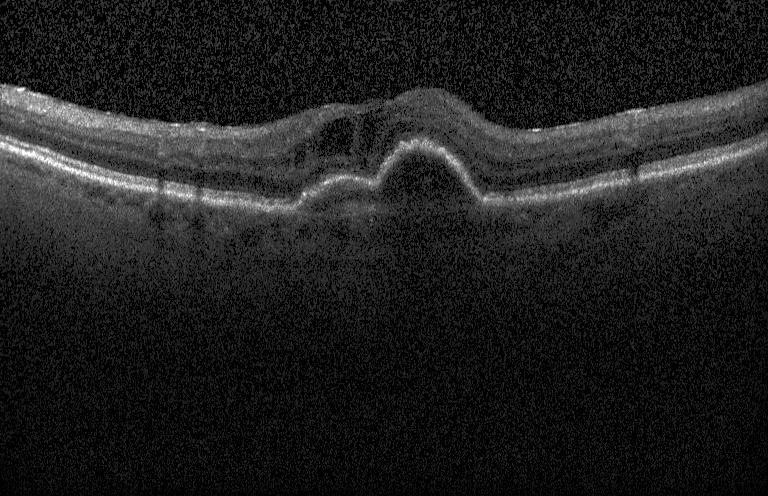
A choroidal neovascular membrane.